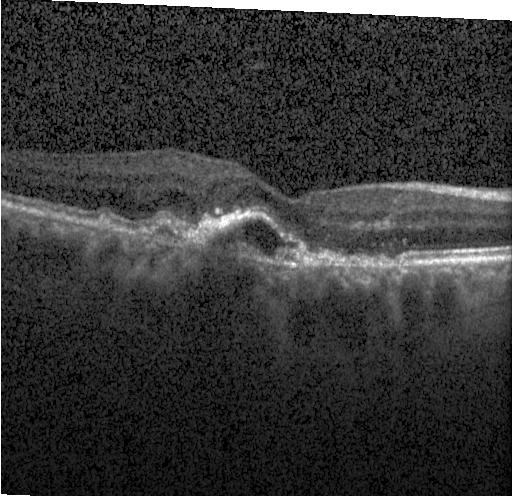 Spectral-domain OCT. OCT line scan
This B-scan demonstrates a choroidal neovascular membrane.